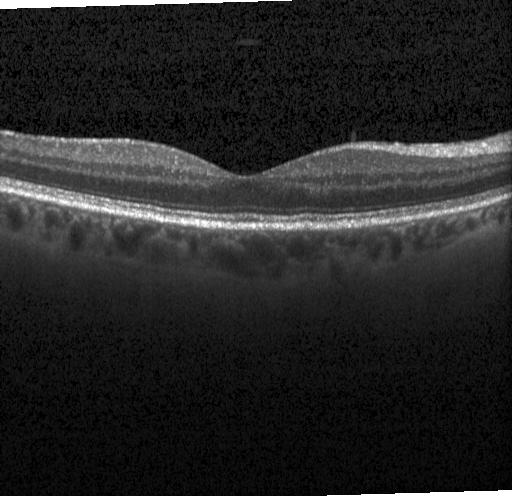
Horizontal scan through the fovea · retinal OCT B-scan · spectral-domain OCT · acquired on a Heidelberg Spectralis.
This B-scan demonstrates neither CNV, DME, nor drusen.